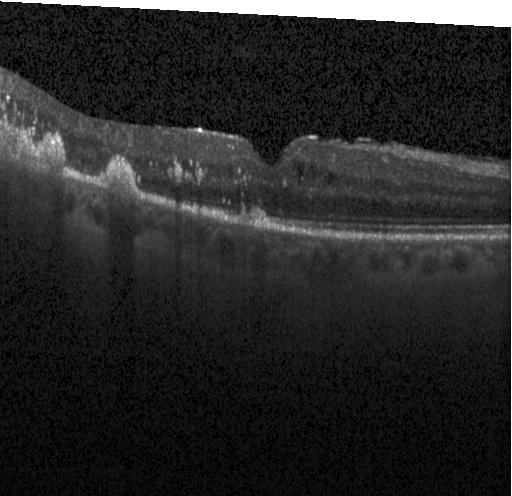

Impression: choroidal neovascularization (CNV).